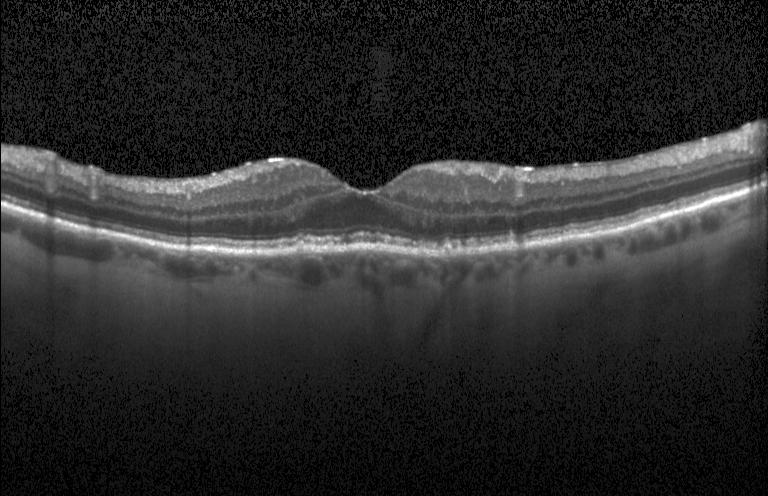

Diagnosis: sub-RPE drusenoid deposits.